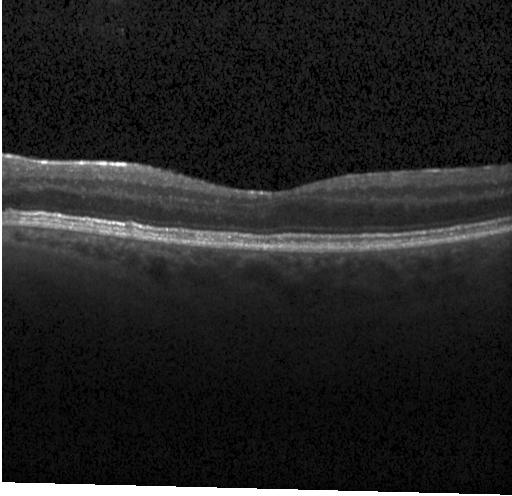
Assessment: no choroidal neovascularization, diabetic macular edema, or drusen.